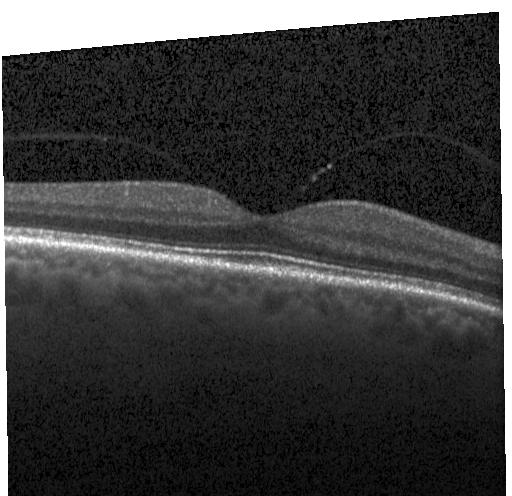
Impression: no evidence of choroidal neovascularization, diabetic macular edema, or drusen.